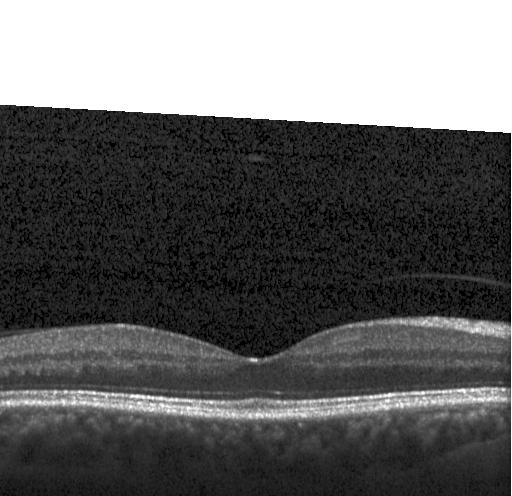 Diagnosis: neither choroidal neovascularization, diabetic macular edema, nor drusen.